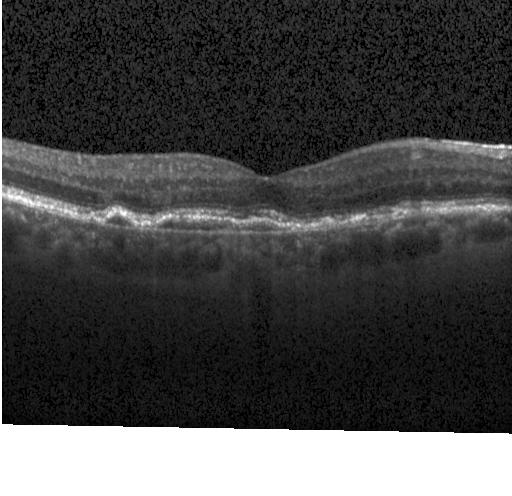 SD-OCT. Centered on the fovea. Instrument: Heidelberg Spectralis. Retinal OCT cross-section — Finding: choroidal neovascularization (CNV).